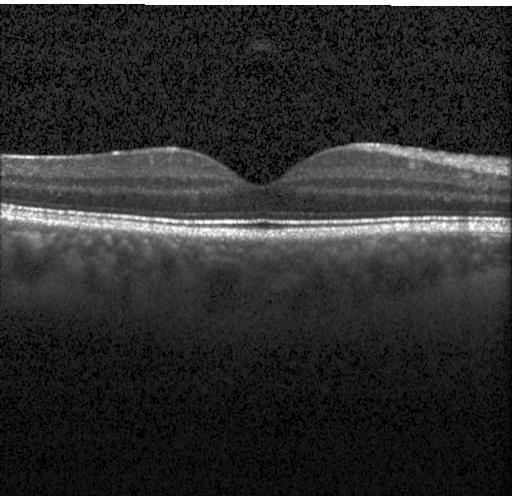
Retinal OCT cross-section showing no choroidal neovascularization, diabetic macular edema, or drusen.